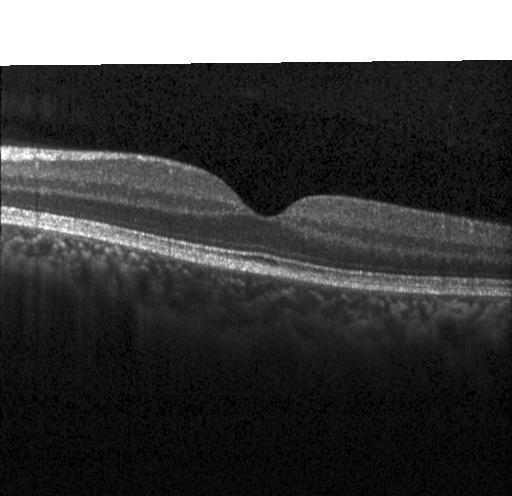 Heidelberg Spectralis OCT system. OCT line scan. SD-OCT. No CNV, no DME, and no drusen.